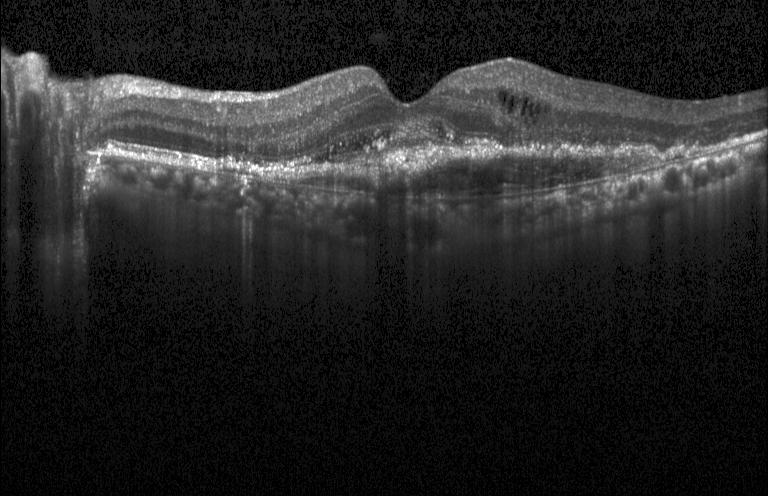
Spectral-domain OCT B-scan: a choroidal neovascular membrane.